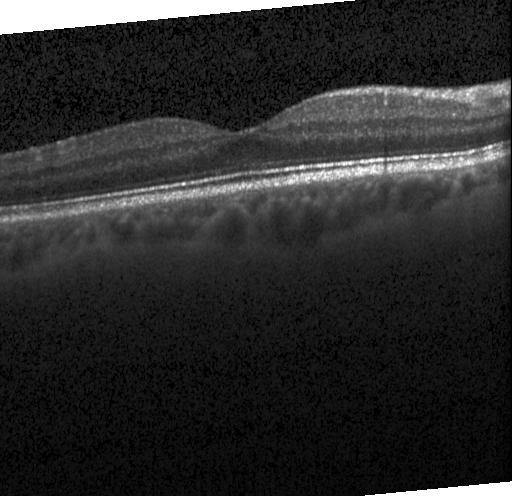 Macular OCT: no choroidal neovascularization, no diabetic macular edema, and no drusen.